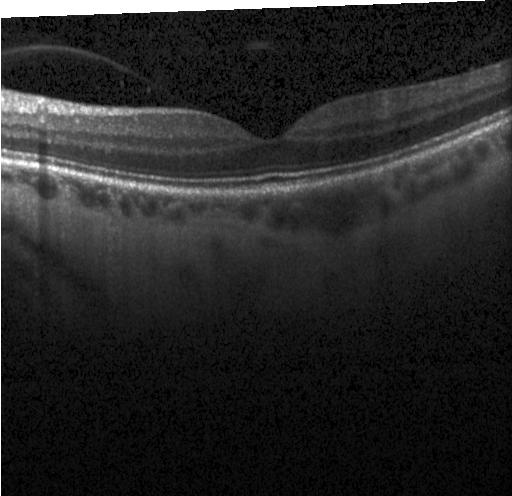

Retinal OCT cross-section.
Assessment: neither choroidal neovascularization, diabetic macular edema, nor drusen.